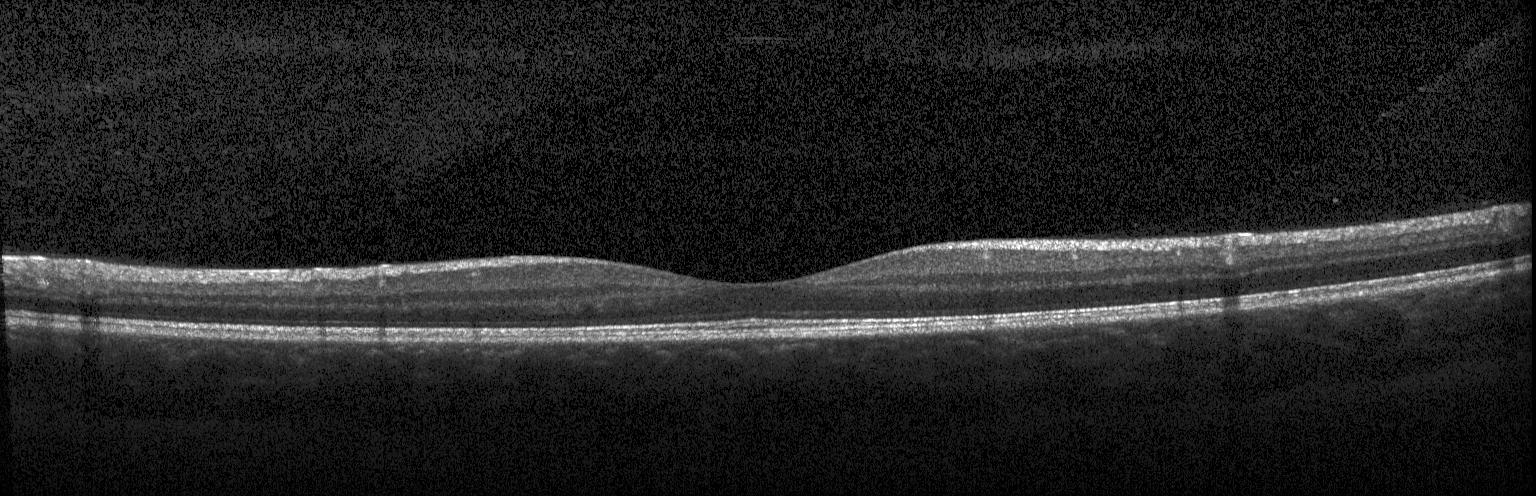
Optical coherence tomography B-scan, through the macula, instrument: Heidelberg Spectralis. No evidence of CNV, DME, or drusen.